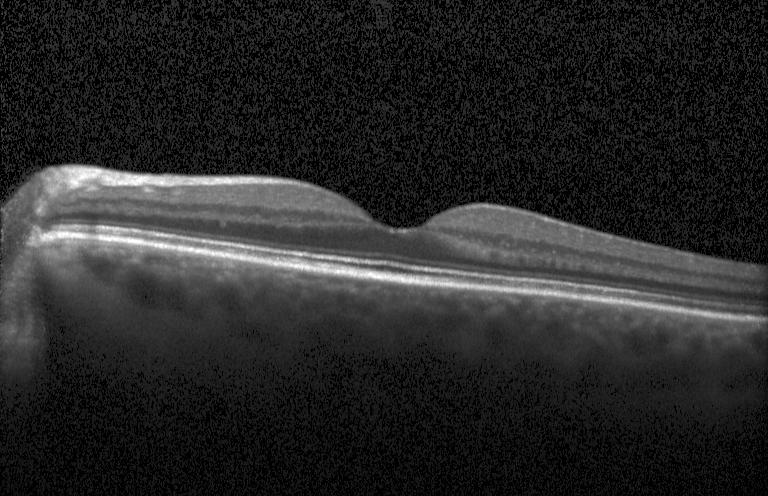
OCT line scan
The scan shows neither choroidal neovascularization, diabetic macular edema, nor drusen.